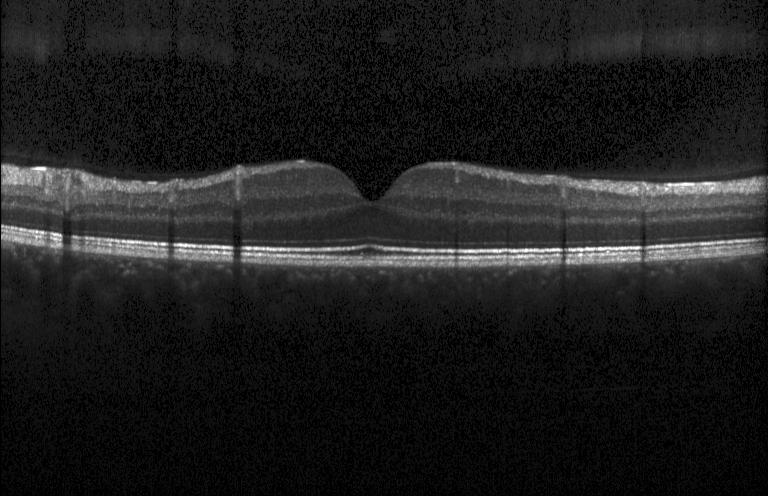
Optical coherence tomography B-scan. Dx: neither choroidal neovascularization, diabetic macular edema, nor drusen.